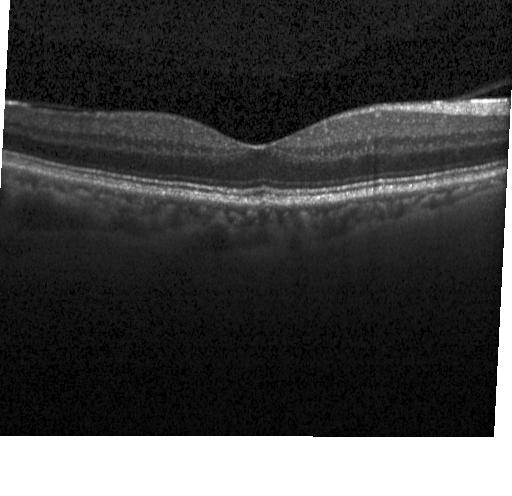
Optical coherence tomography B-scan. Heidelberg Spectralis. Spectral-domain OCT. Fovea-centered.
Impression: no choroidal neovascularization, diabetic macular edema, or drusen.